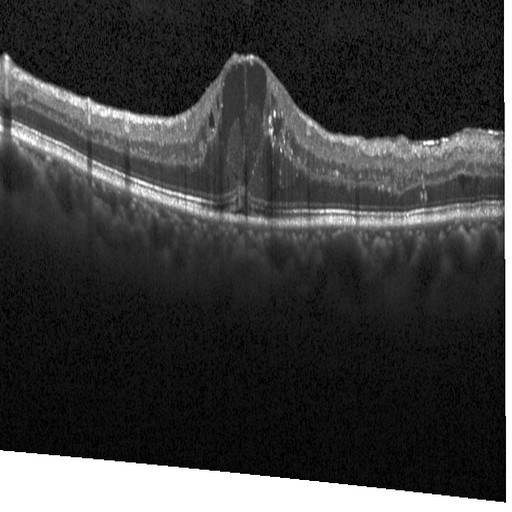

Through the macula; Heidelberg Spectralis; optical coherence tomography B-scan; spectral-domain optical coherence tomography.
Finding: diabetic macular edema (DME).